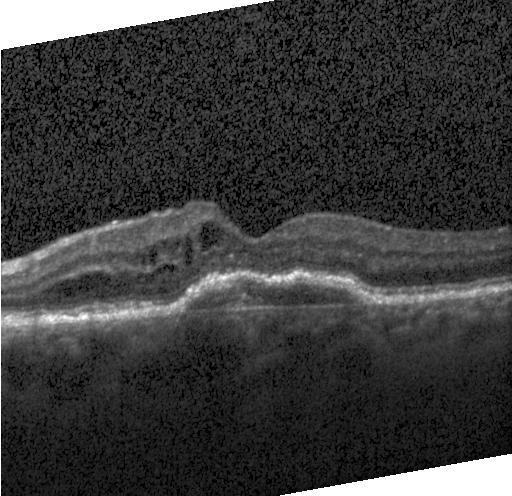 Instrument: Heidelberg Spectralis · OCT B-scan · spectral-domain OCT · horizontal scan through the fovea. The scan shows a choroidal neovascular membrane.